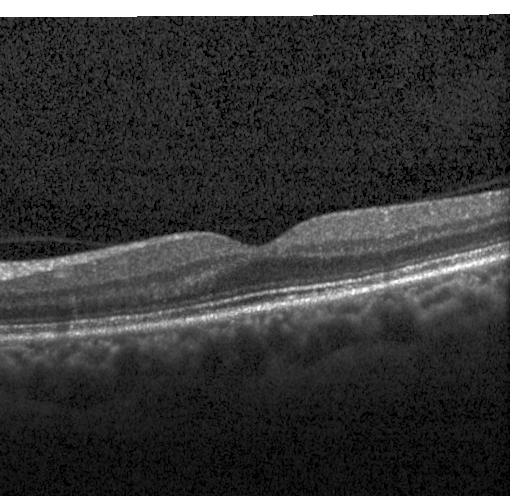 Retinal OCT B-scan.
Impression: no CNV, no DME, and no drusen.